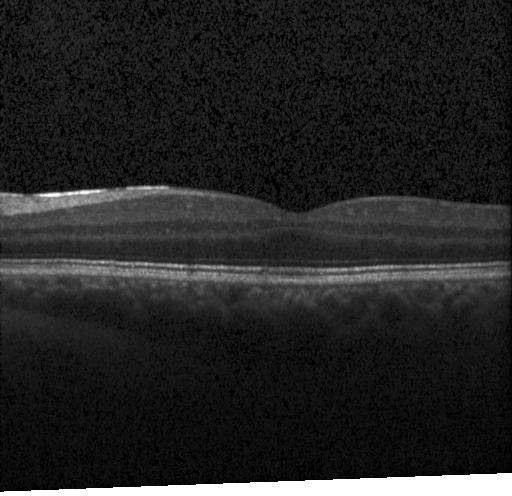 Macular OCT demonstrating no CNV, DME, or drusen.